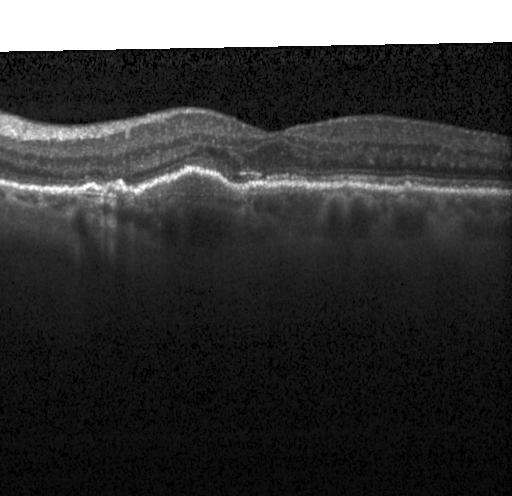 Impression: choroidal neovascularization (CNV).